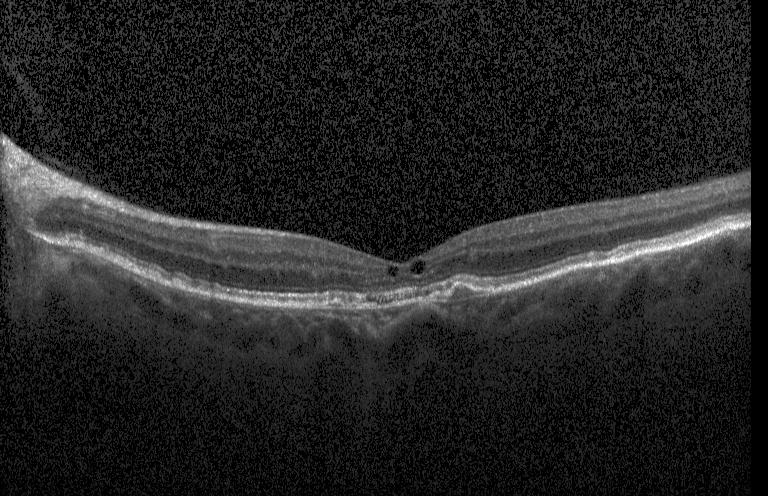

Through the macula. Heidelberg Spectralis. Optical coherence tomography scan. Spectral-domain OCT.
Finding: a choroidal neovascular membrane.